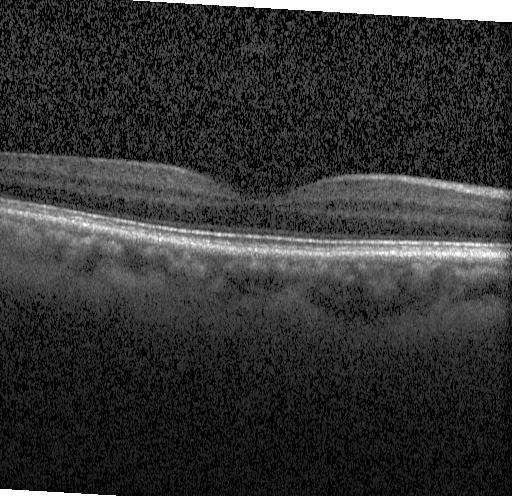
Spectral-domain OCT · OCT B-scan · centered on the fovea · acquired on a Heidelberg Spectralis — Impression: no CNV, DME, or drusen.